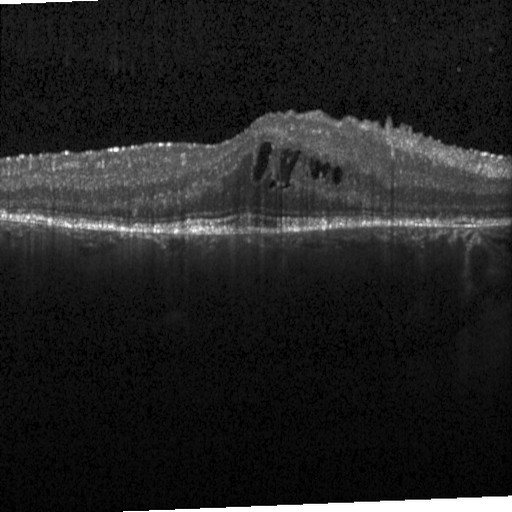 Diagnosis: diabetic macular edema.